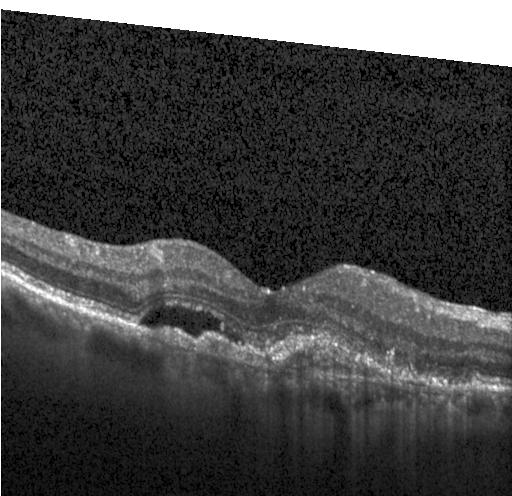 Retinal OCT cross-section; spectral-domain OCT
Diagnosis: choroidal neovascularization.